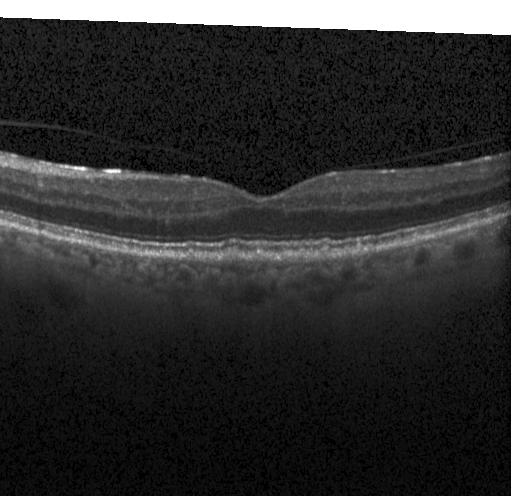 OCT line scan. Spectral-domain OCT. The scan shows sub-RPE drusenoid deposits.